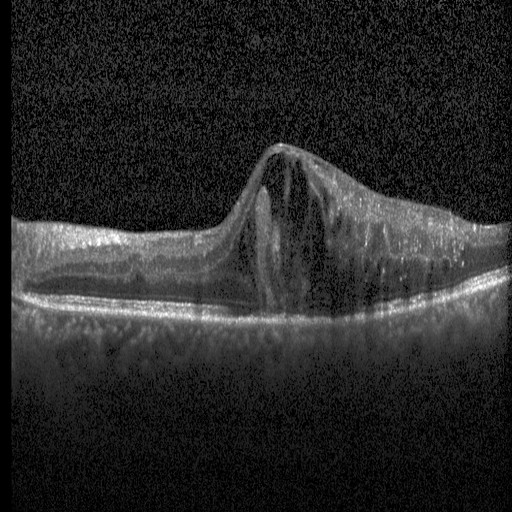

SD-OCT; through the macula; optical coherence tomography scan; Heidelberg Spectralis OCT system.
Assessment: diabetic macular edema.